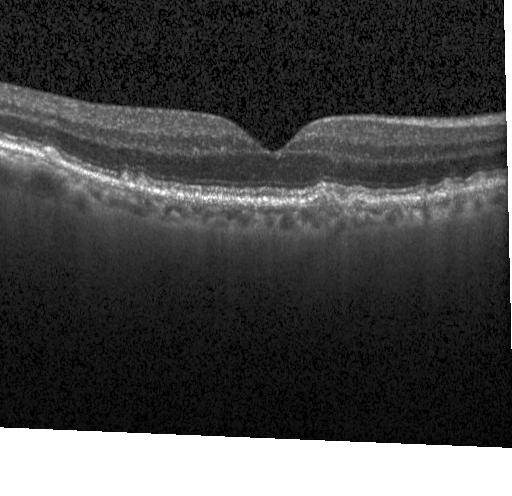
Heidelberg Spectralis OCT system · macular scan · spectral-domain OCT · optical coherence tomography scan — The scan shows multiple drusen.